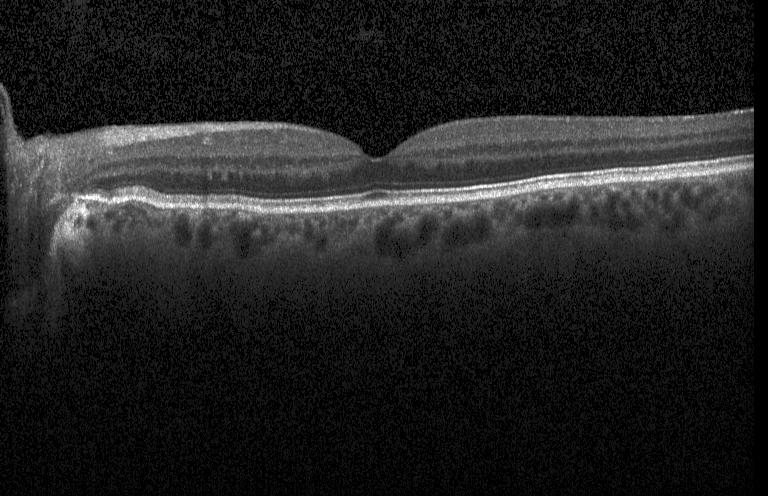
No choroidal neovascularization, no diabetic macular edema, and no drusen.